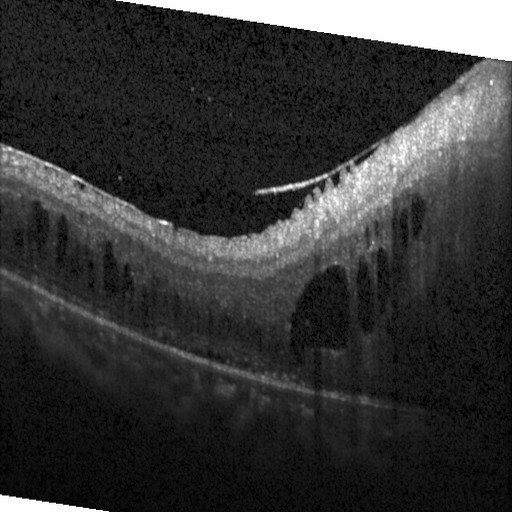
Macular OCT: diabetic macular edema.